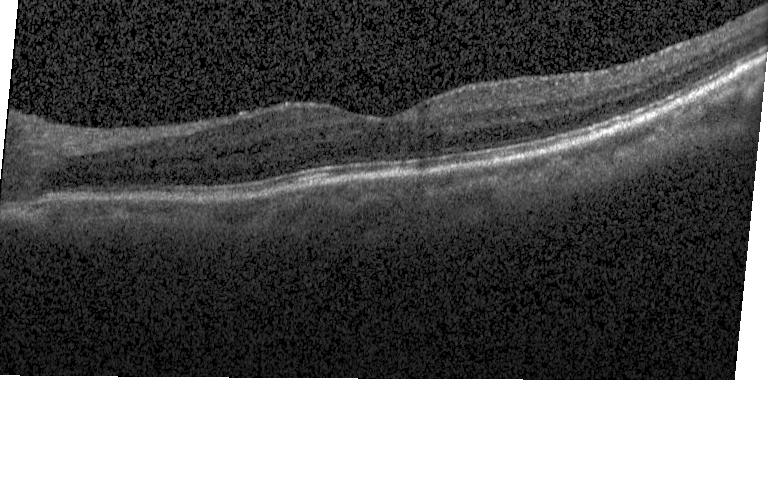
OCT line scan.
This B-scan demonstrates no evidence of choroidal neovascularization, diabetic macular edema, or drusen.